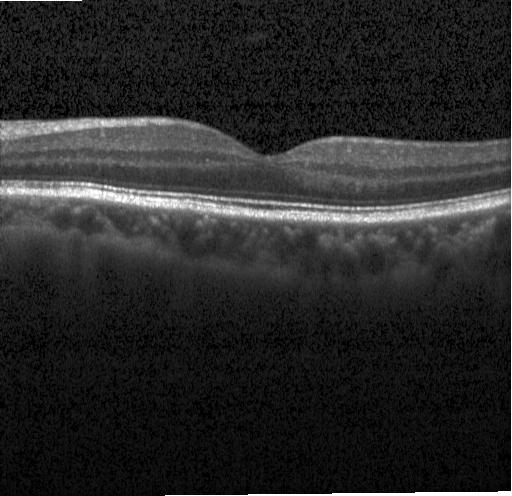 OCT line scan · instrument: Heidelberg Spectralis · through the macula
No CNV, DME, or drusen.